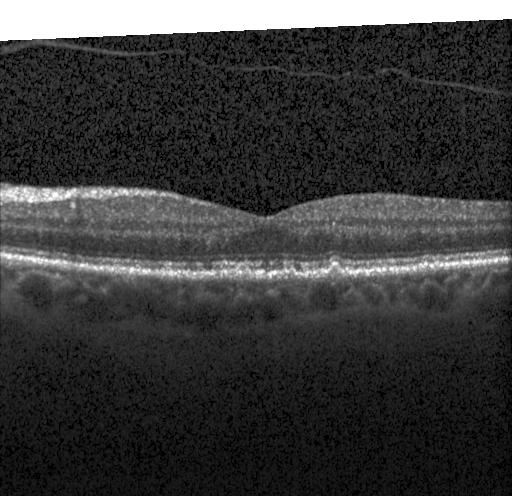 Heidelberg Spectralis OCT system; fovea-centered; OCT line scan. Impression: drusen.